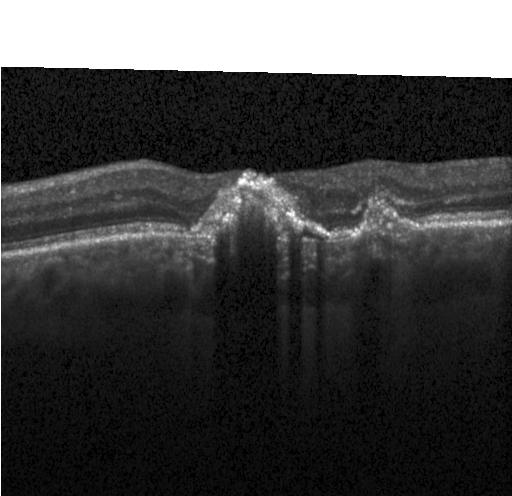 Macular OCT demonstrating CNV.